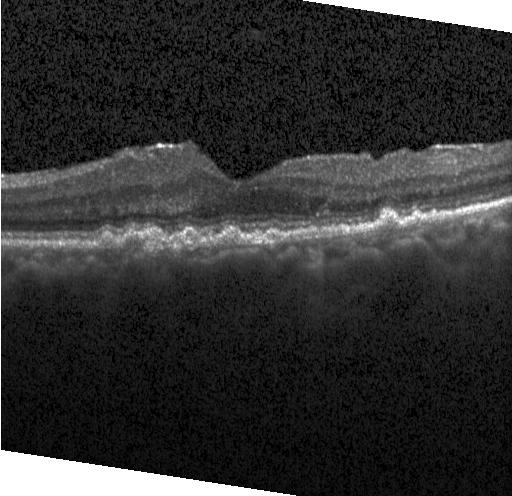 OCT line scan — Multiple drusen.